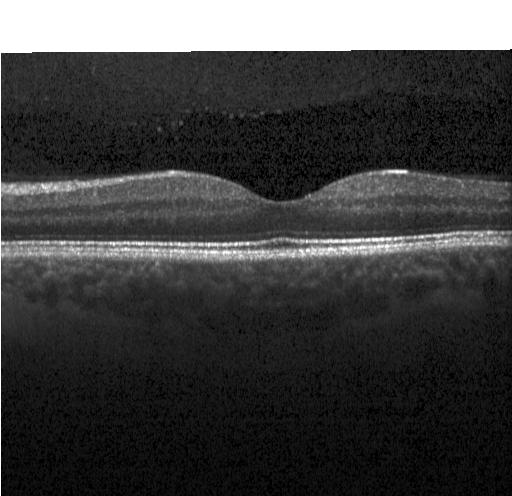 SD-OCT. Optical coherence tomography B-scan. Centered on the fovea. Instrument: Heidelberg Spectralis — This B-scan demonstrates no CNV, no DME, and no drusen.